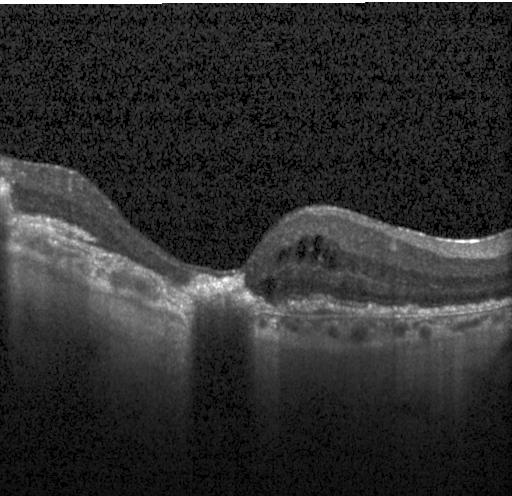 Heidelberg Spectralis; retinal OCT cross-section. This B-scan demonstrates choroidal neovascularization (CNV).